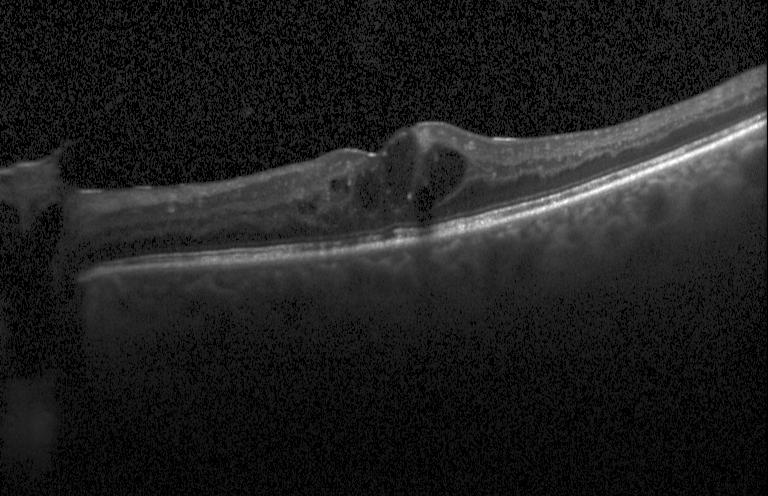 Diagnosis: diabetic macular edema.